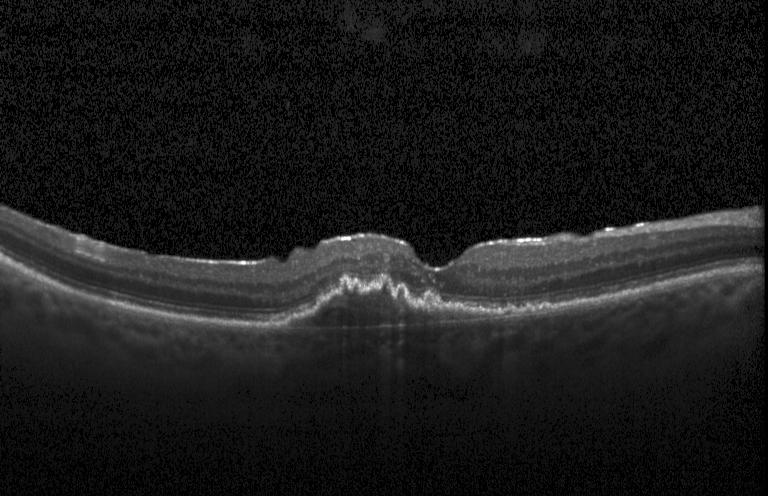 Fovea-centered. OCT B-scan. Spectral-domain OCT. Heidelberg Spectralis OCT system.
Impression: a choroidal neovascular membrane.